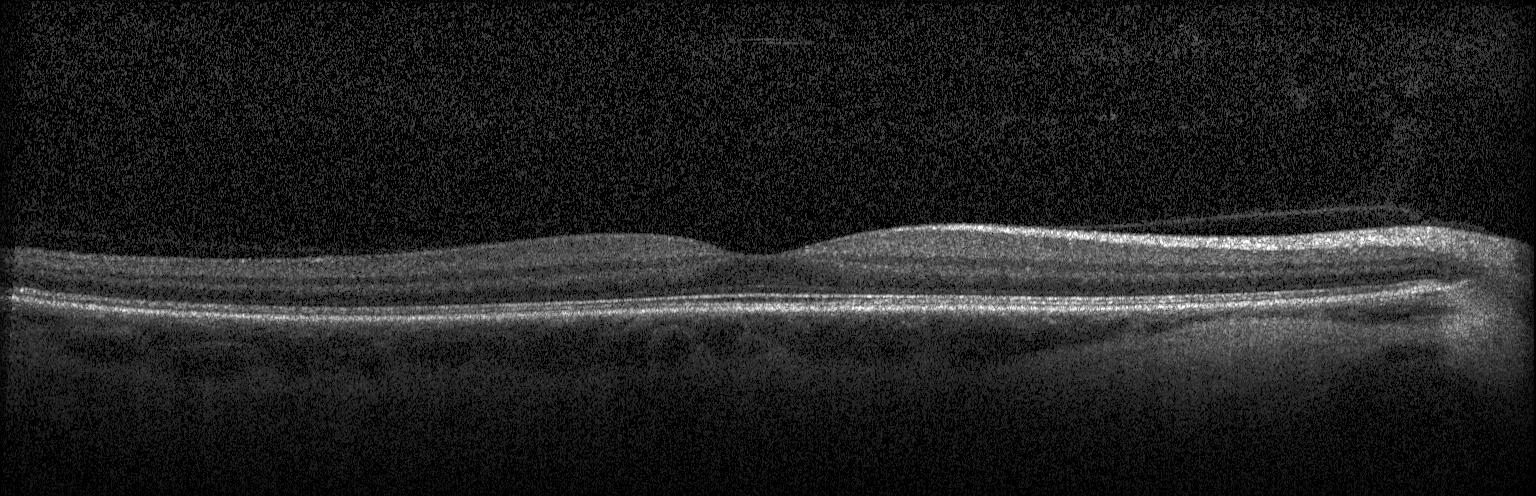 Retinal OCT B-scan, spectral-domain optical coherence tomography, instrument: Heidelberg Spectralis.
Impression: no CNV, DME, or drusen.